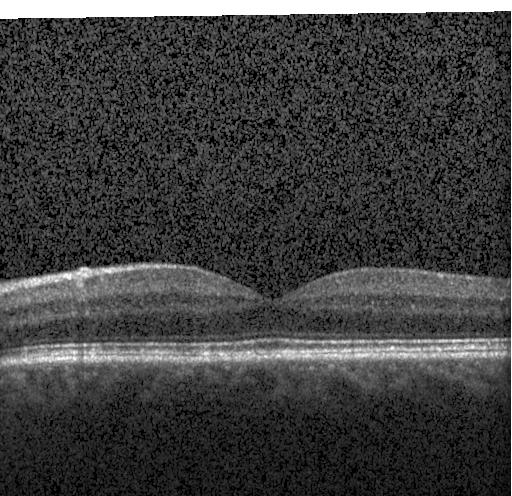

Retinal OCT cross-section showing no choroidal neovascularization, diabetic macular edema, or drusen.